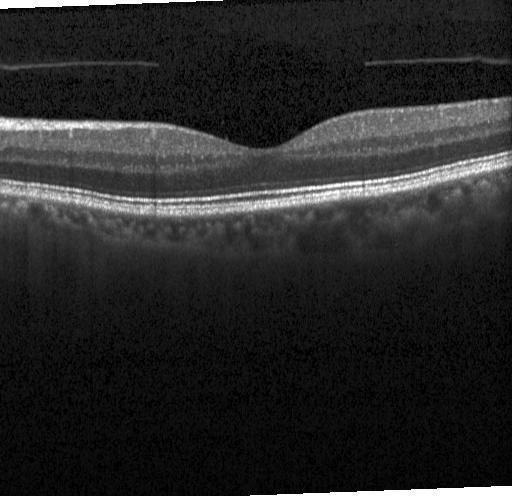
Centered on the fovea, OCT line scan.
Finding: no CNV, DME, or drusen.